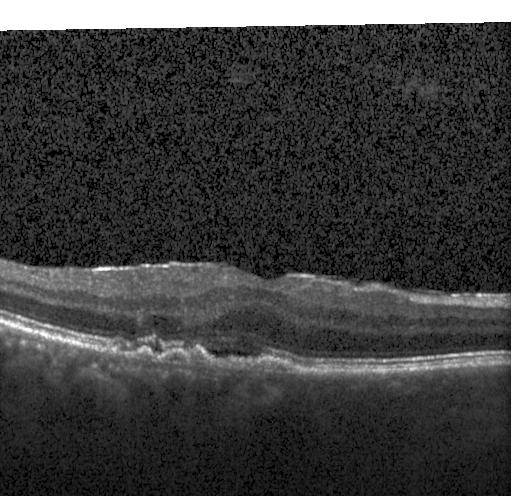 Finding: CNV.